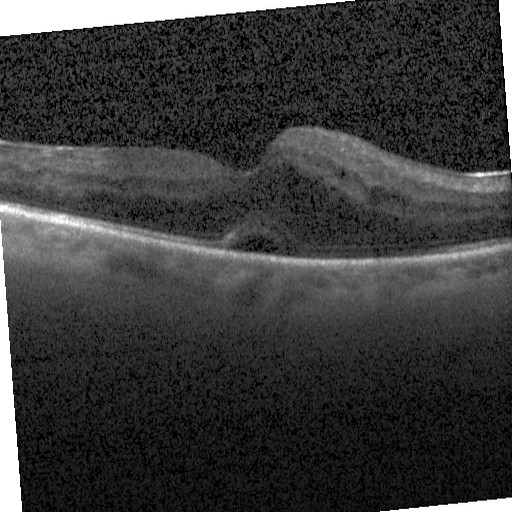
Retinal OCT cross-section showing DME.